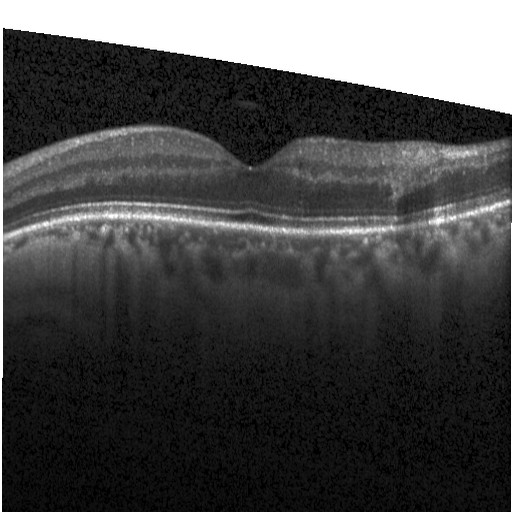 Spectral-domain OCT B-scan: diabetic macular edema.